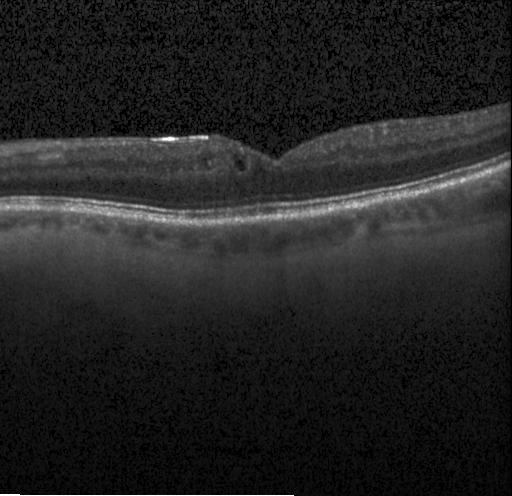

Optical coherence tomography B-scan. Fovea-centered — Dx: diabetic macular edema.